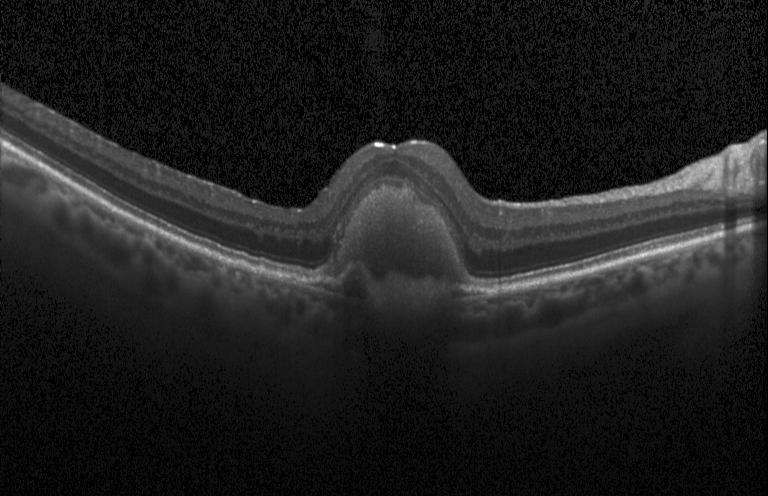

OCT line scan
The scan shows a choroidal neovascular membrane.